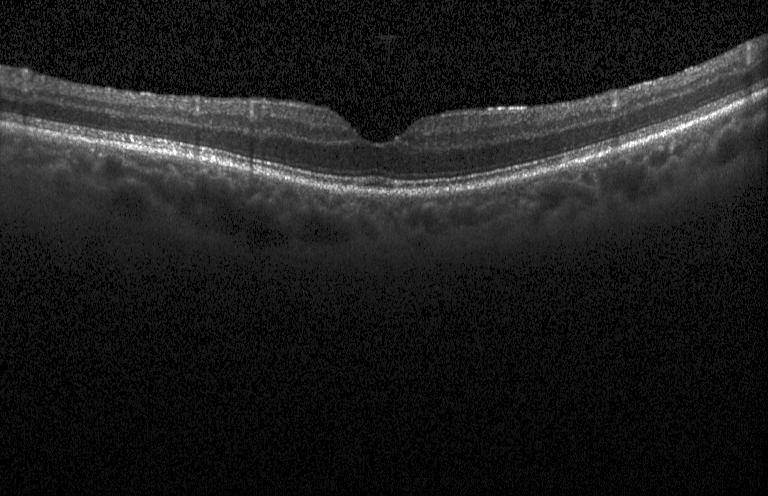

OCT line scan. OCT finding: no evidence of choroidal neovascularization, diabetic macular edema, or drusen.